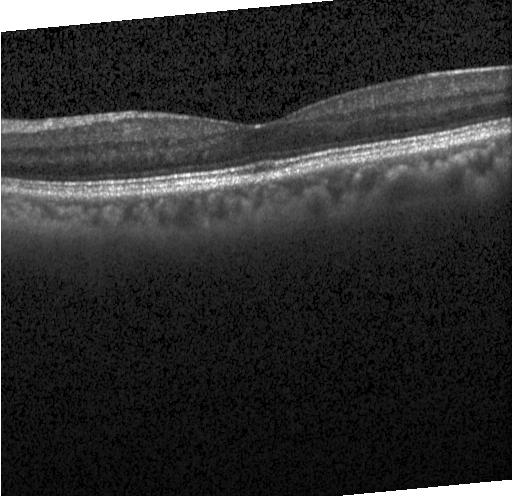 The scan shows no choroidal neovascularization, no diabetic macular edema, and no drusen.